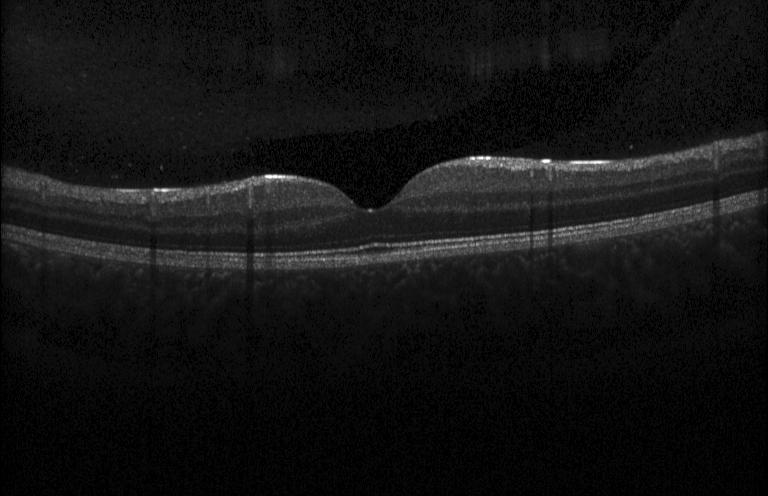

Through the macula; retinal OCT B-scan — The scan shows neither choroidal neovascularization, diabetic macular edema, nor drusen.